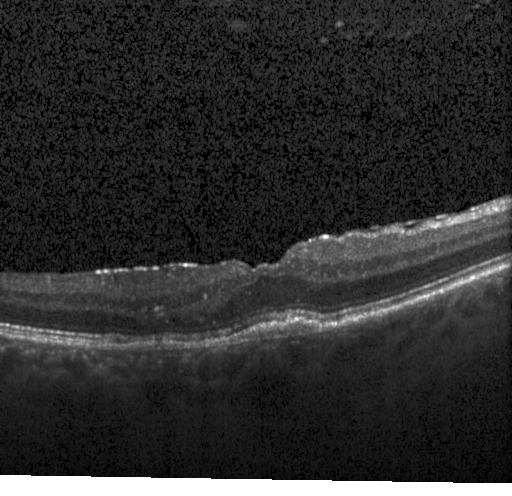 Spectral-domain OCT · retinal OCT B-scan
This B-scan demonstrates a choroidal neovascular membrane.